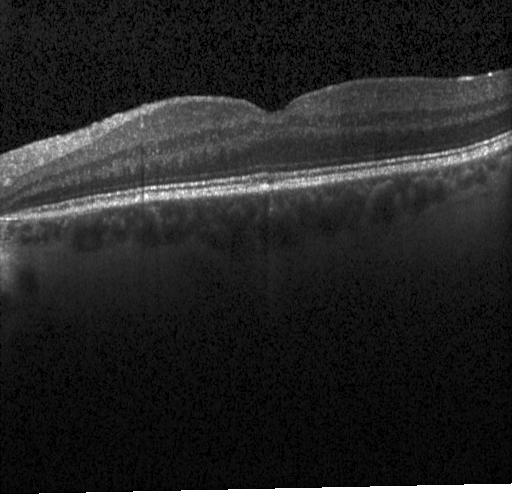

The scan shows no choroidal neovascularization, no diabetic macular edema, and no drusen.